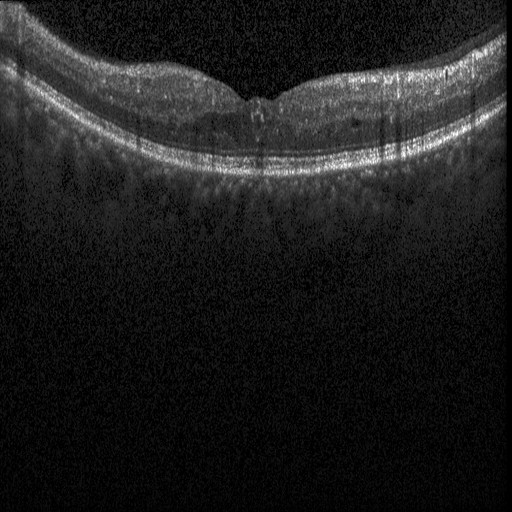
Dx: DME.